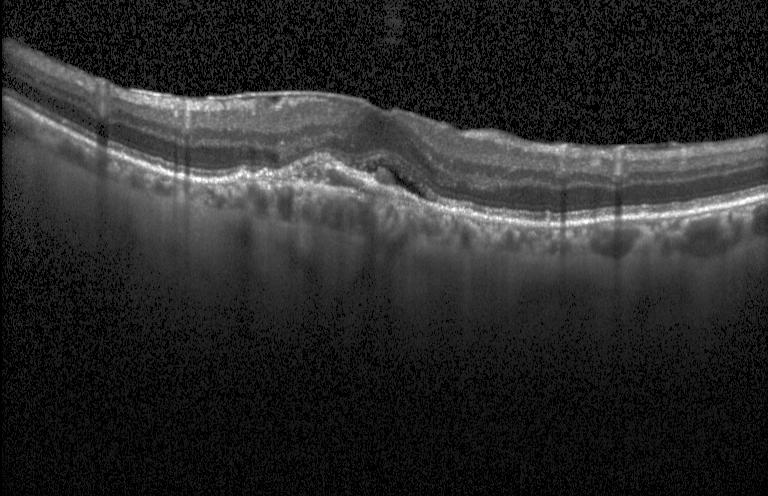 Retinal OCT cross-section; acquired on a Heidelberg Spectralis. Assessment: a choroidal neovascular membrane.